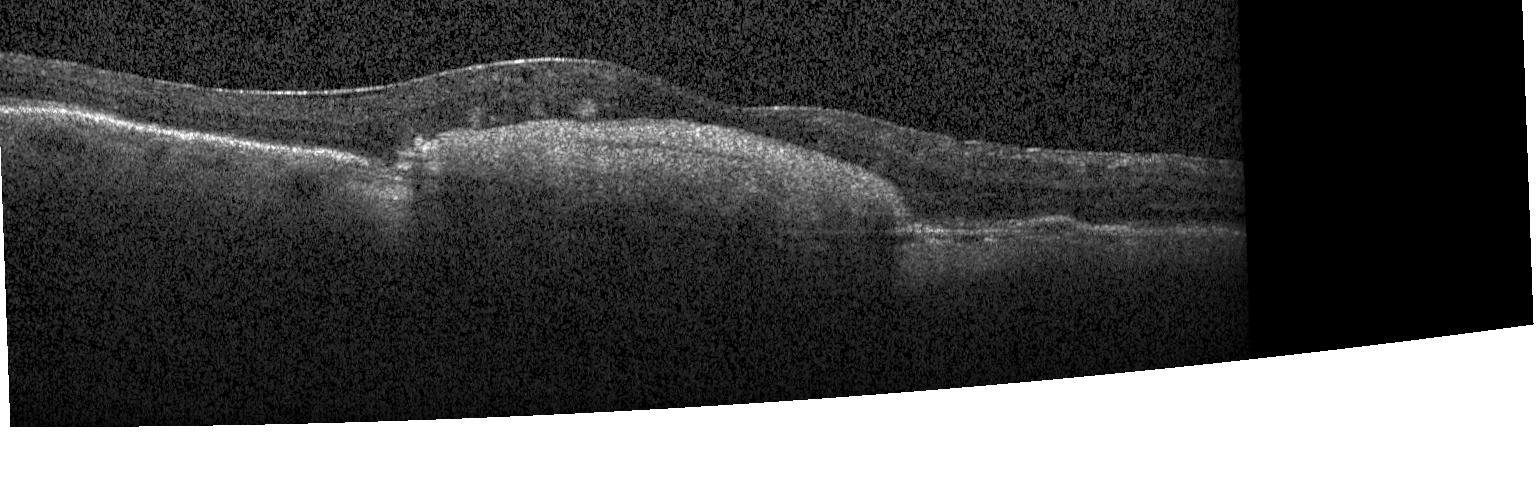

Optical coherence tomography scan · spectral-domain optical coherence tomography
Diagnosis: a choroidal neovascular membrane.